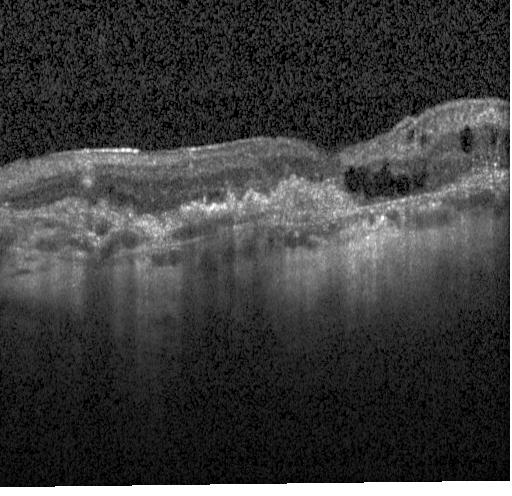
OCT finding: a choroidal neovascular membrane.